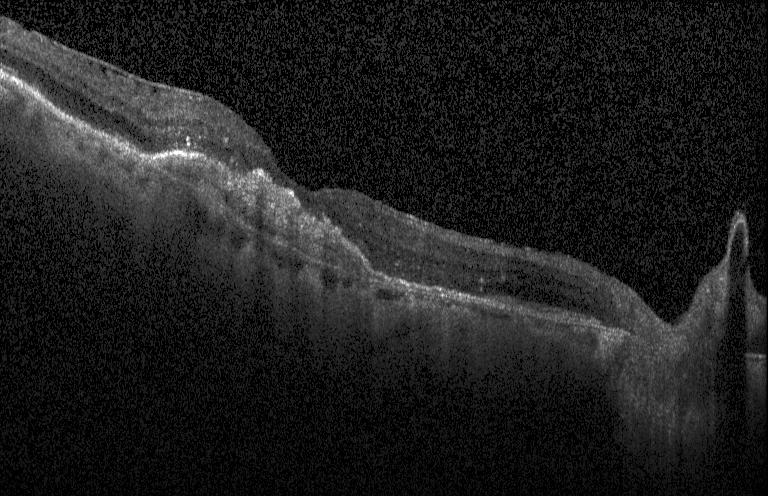 Impression: CNV.